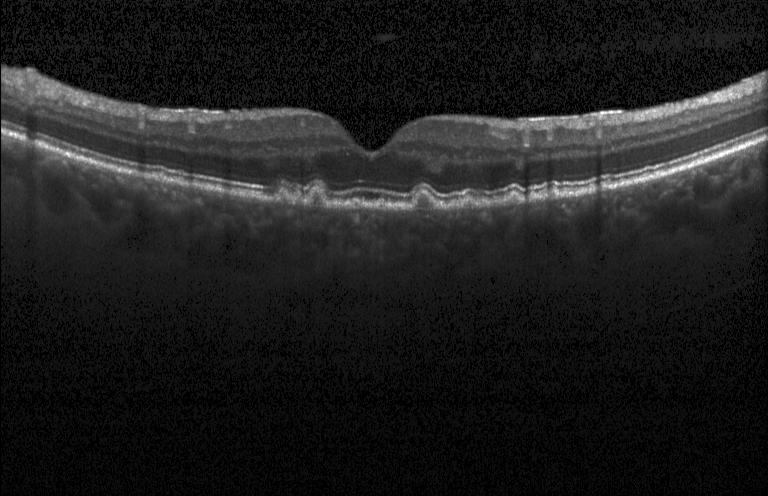 OCT finding: multiple drusen.